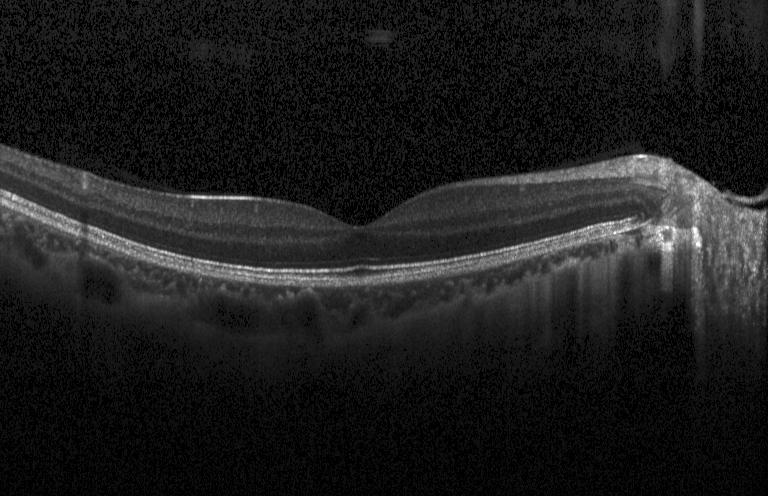

Neither choroidal neovascularization, diabetic macular edema, nor drusen.